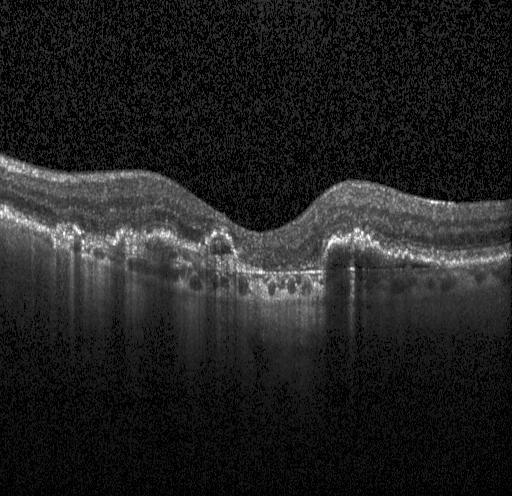

Fovea-centered; SD-OCT; optical coherence tomography scan; Heidelberg Spectralis OCT system — Diagnosis: choroidal neovascularization.